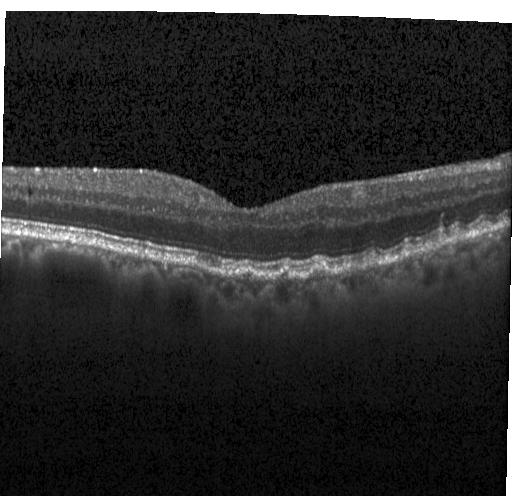

Optical coherence tomography scan, acquired on a Heidelberg Spectralis
Finding: drusen.